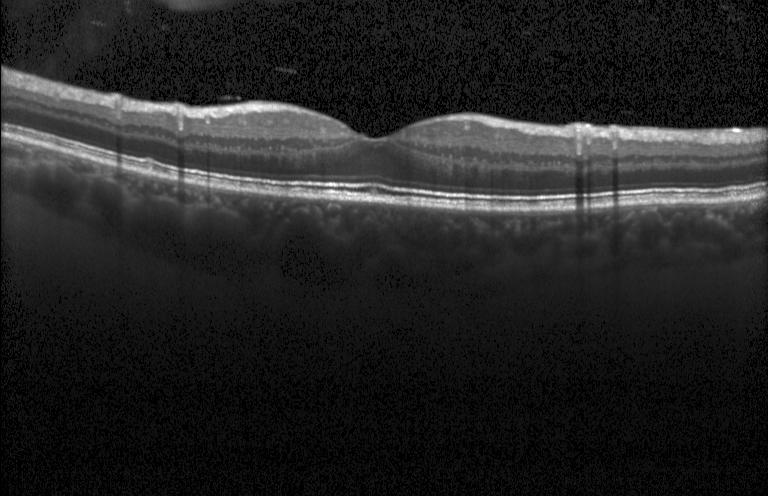

Heidelberg Spectralis OCT system; SD-OCT; macular scan; OCT line scan.
The scan shows neither CNV, DME, nor drusen.